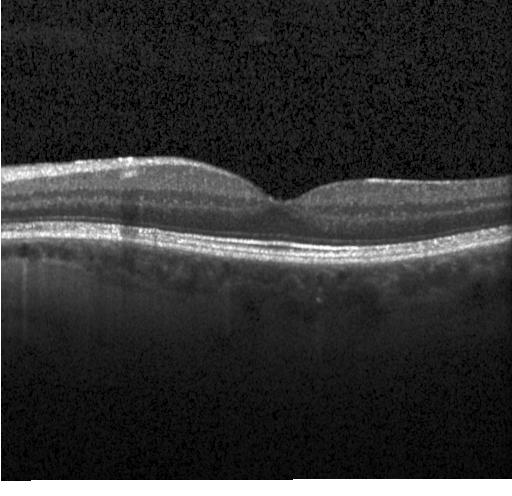

Optical coherence tomography scan. Spectral-domain OCT.
The scan shows no choroidal neovascularization, diabetic macular edema, or drusen.